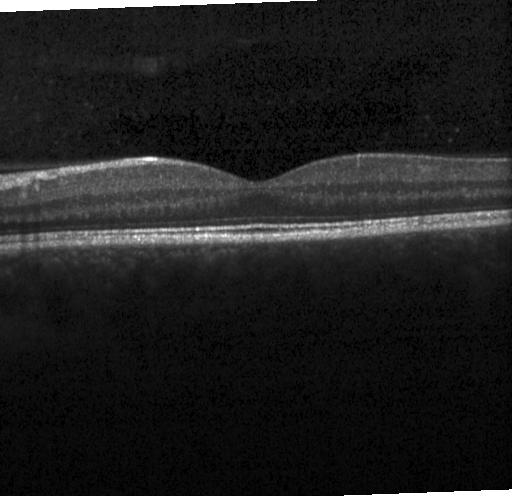

Retinal OCT cross-section. No choroidal neovascularization, no diabetic macular edema, and no drusen.